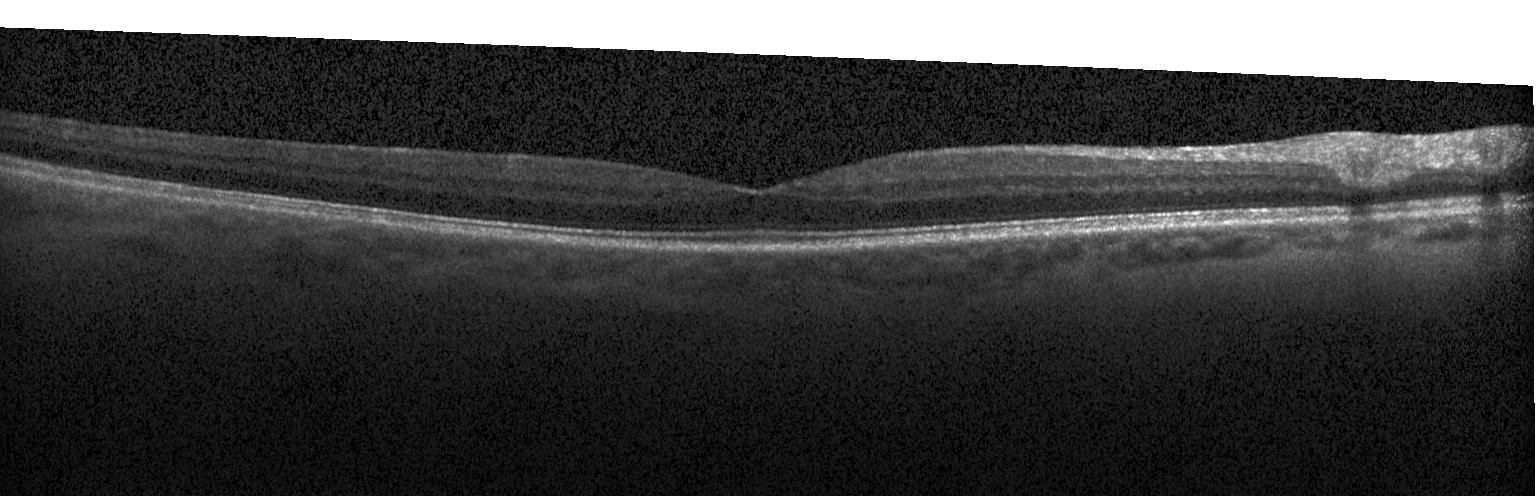 Retinal OCT cross-section showing neither choroidal neovascularization, diabetic macular edema, nor drusen.